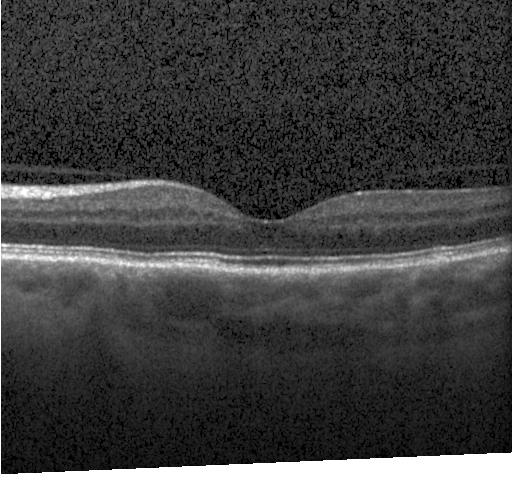

Finding: neither choroidal neovascularization, diabetic macular edema, nor drusen.